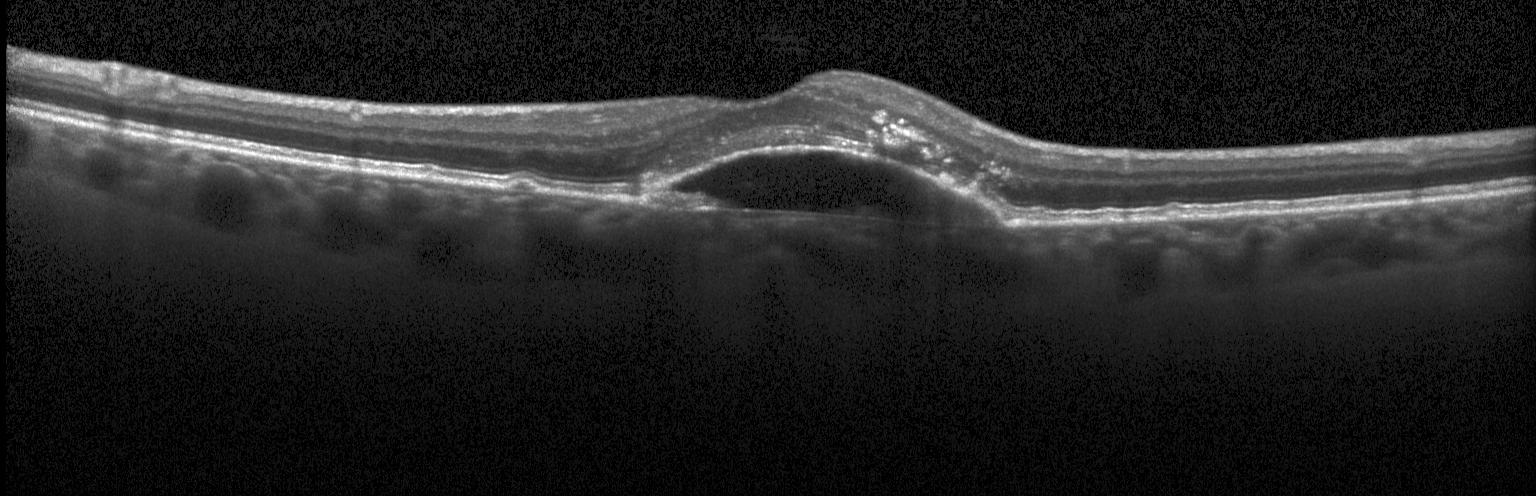
Optical coherence tomography B-scan.
Diagnosis: a choroidal neovascular membrane.